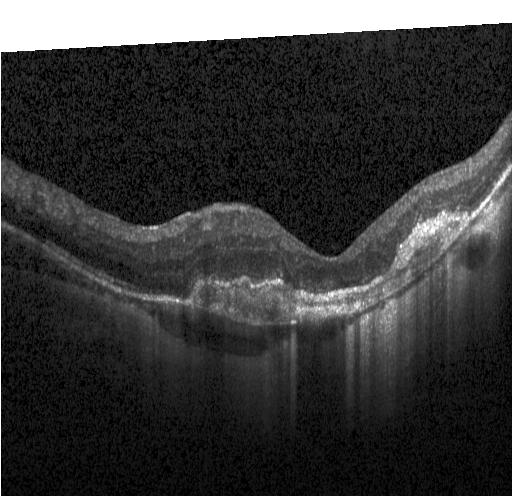 OCT B-scan showing a choroidal neovascular membrane.